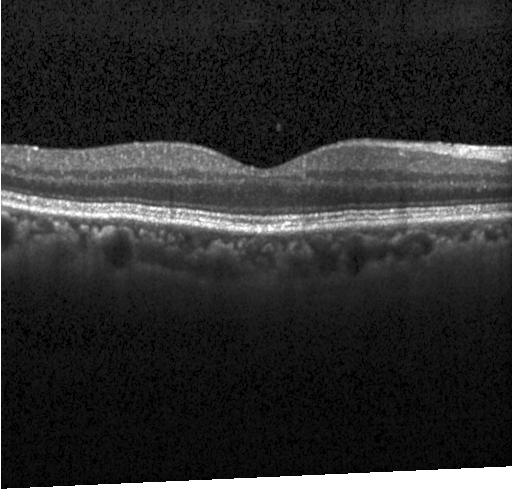 Macular OCT demonstrating no evidence of choroidal neovascularization, diabetic macular edema, or drusen.